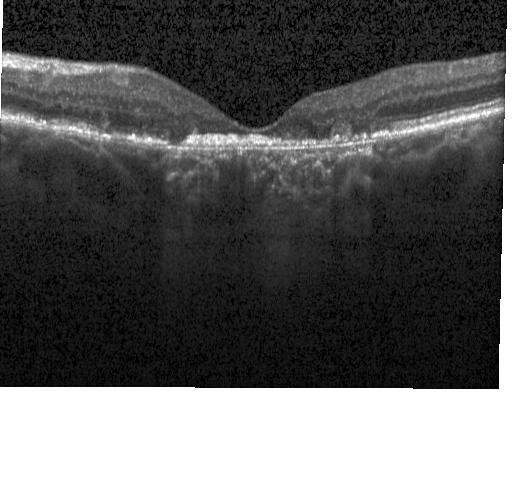 OCT B-scan.
Impression: choroidal neovascularization (CNV).